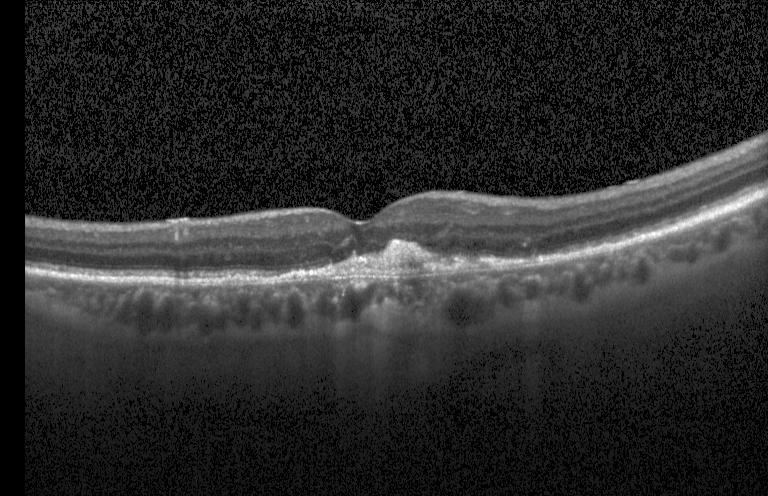 Spectral-domain OCT · Heidelberg Spectralis OCT system · optical coherence tomography B-scan. Diagnosis: choroidal neovascularization (CNV).